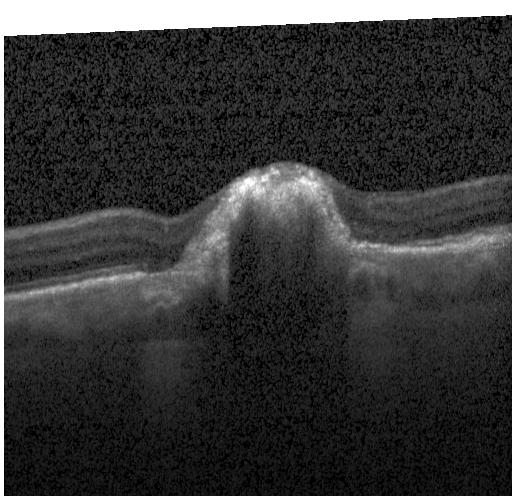

OCT scan showing choroidal neovascularization (CNV).